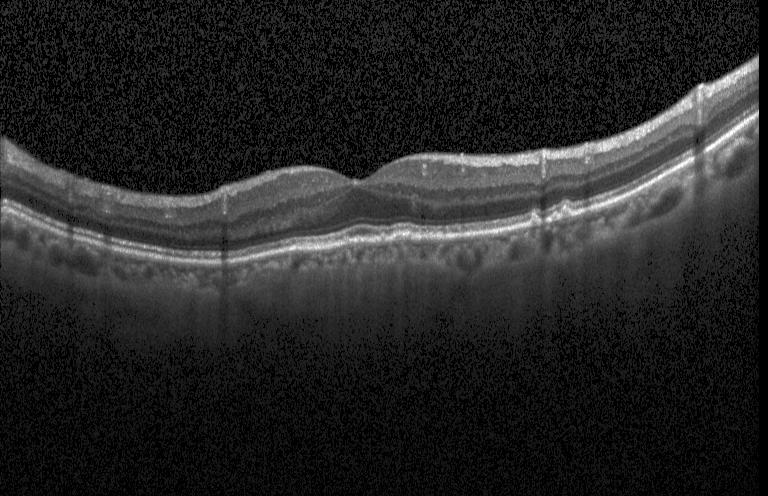

OCT B-scan showing drusen.